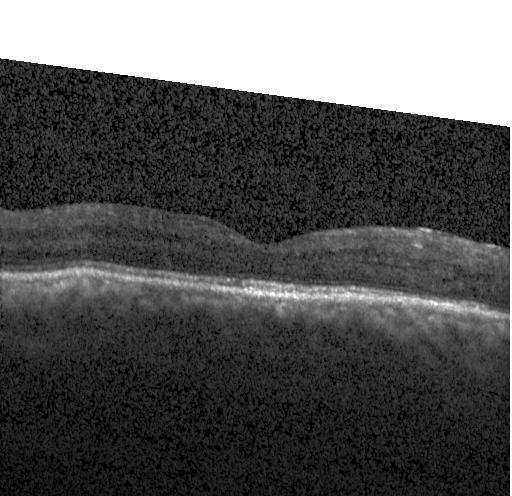 Retinal OCT B-scan.
OCT finding: no CNV, no DME, and no drusen.